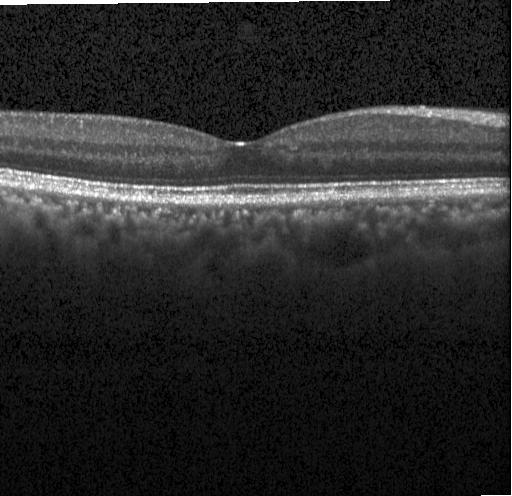
Spectral-domain OCT; OCT line scan.
Finding: neither choroidal neovascularization, diabetic macular edema, nor drusen.